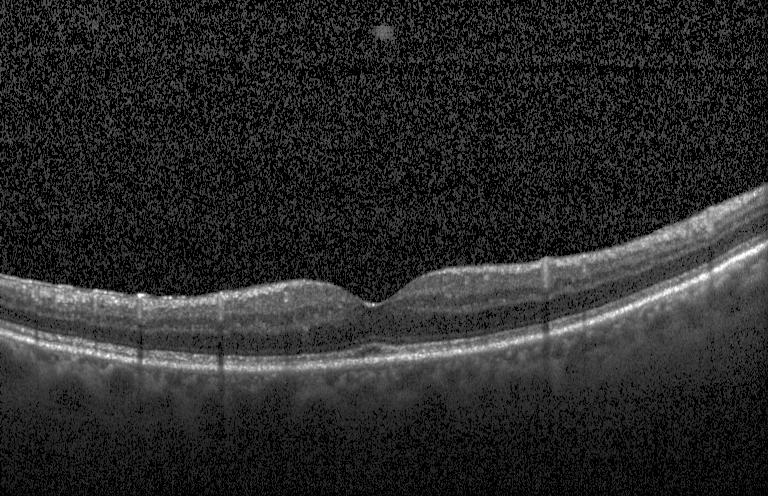

Centered on the fovea. Spectral-domain OCT. OCT B-scan. Heidelberg Spectralis OCT system — Finding: no choroidal neovascularization, no diabetic macular edema, and no drusen.